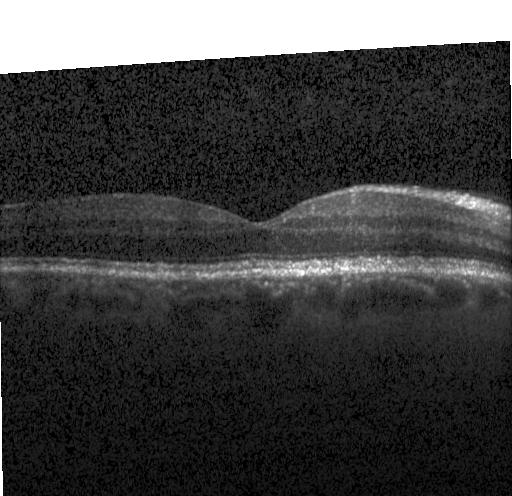

Retinal OCT cross-section showing no CNV, no DME, and no drusen.